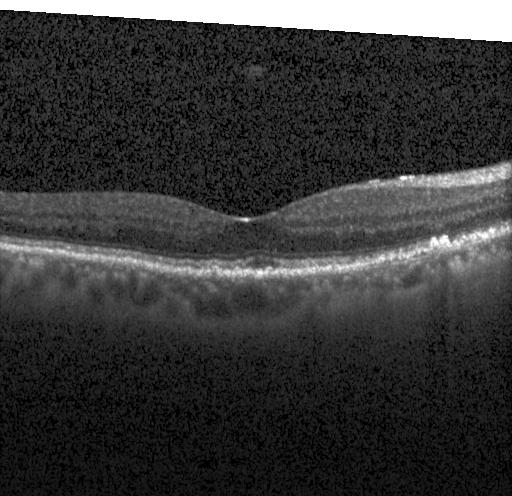 Macular OCT: drusen.